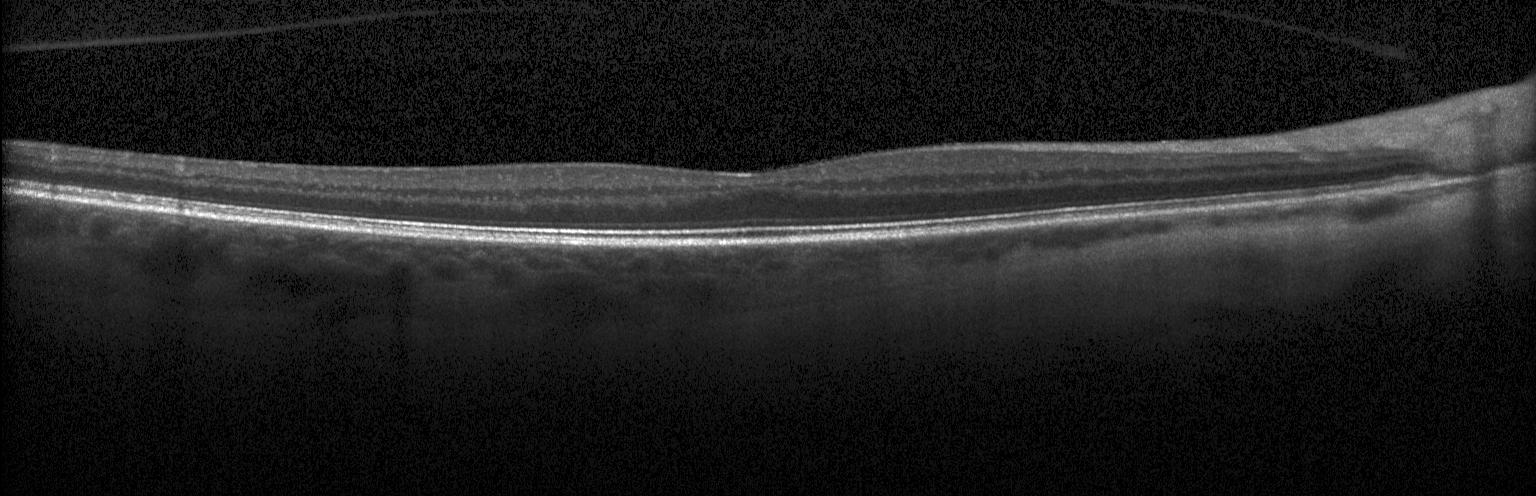
OCT line scan
Impression: no evidence of CNV, DME, or drusen.